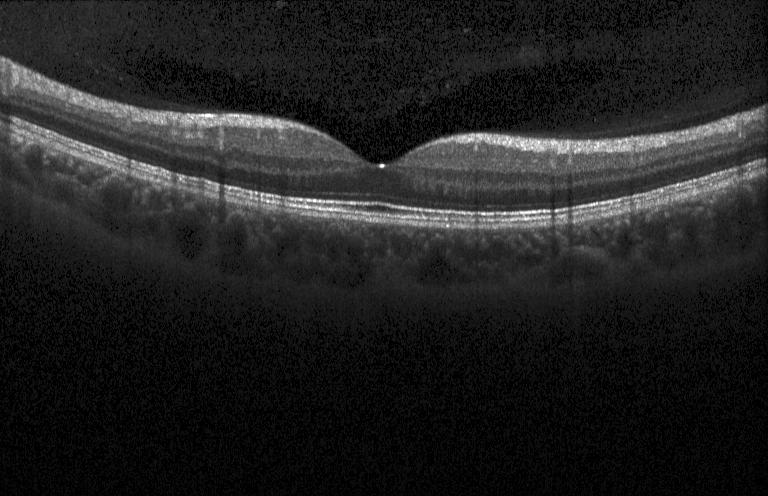 Retinal OCT cross-section — Macular OCT: no choroidal neovascularization, no diabetic macular edema, and no drusen.